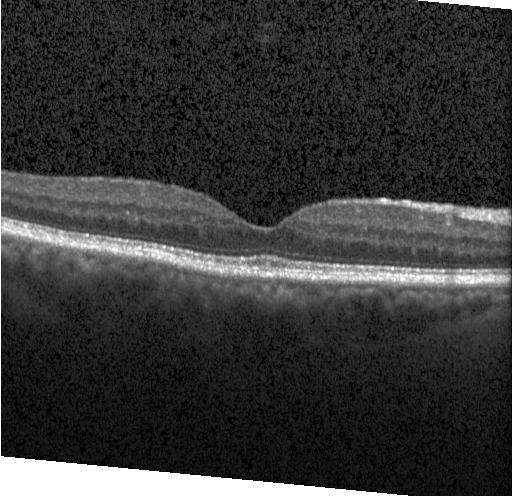 Horizontal scan through the fovea; spectral-domain OCT; acquired on a Heidelberg Spectralis; OCT line scan — Assessment: neither choroidal neovascularization, diabetic macular edema, nor drusen.